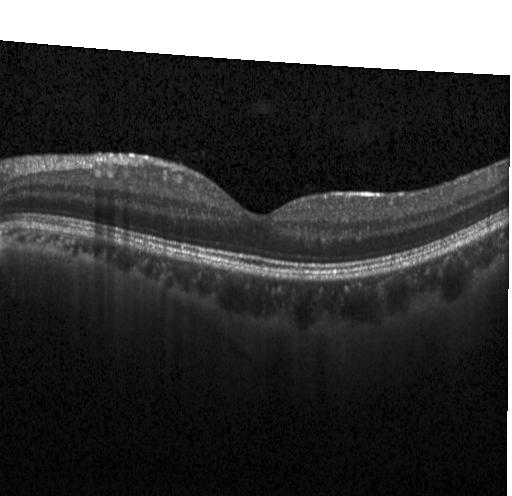
Retinal OCT cross-section showing no CNV, no DME, and no drusen.